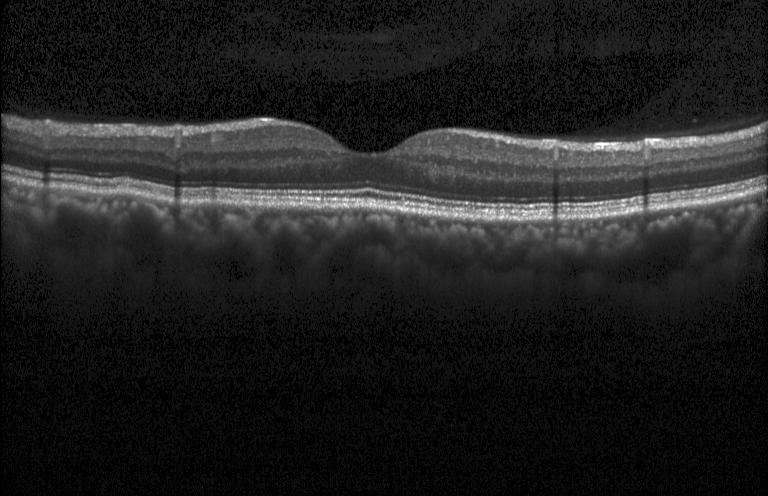 OCT finding: neither choroidal neovascularization, diabetic macular edema, nor drusen.